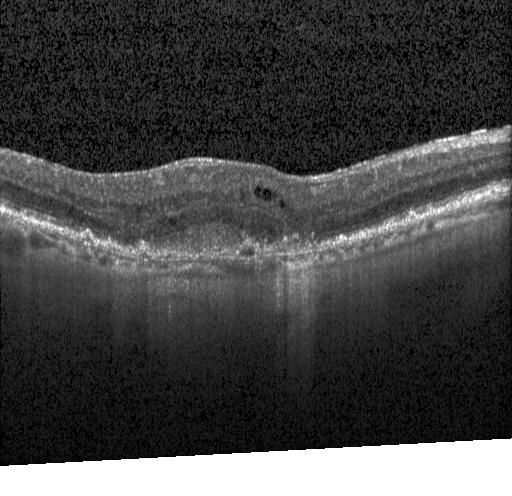

Finding: CNV.